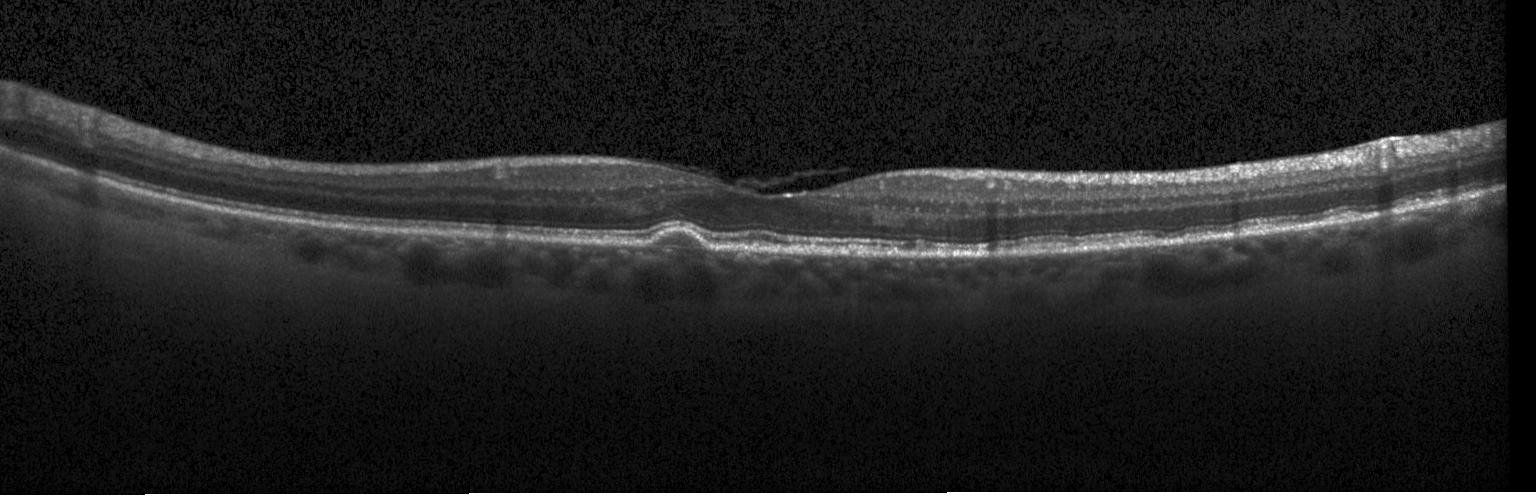
Retinal OCT cross-section. Fovea-centered
Impression: multiple drusen.